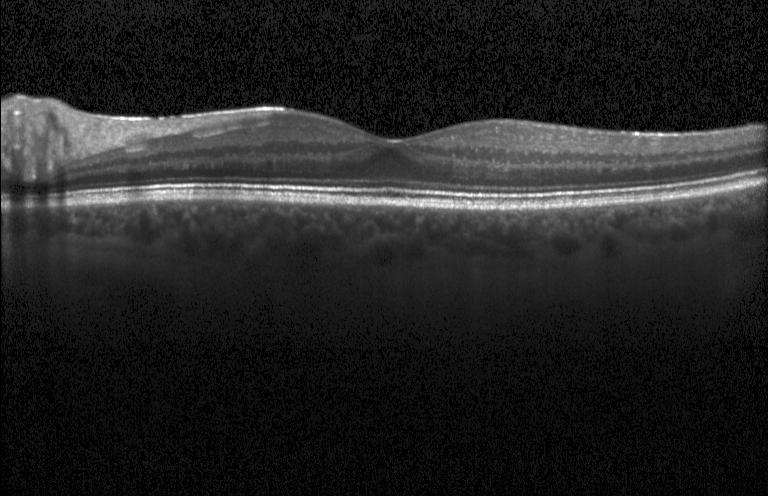

SD-OCT; horizontal scan through the fovea; optical coherence tomography B-scan; Heidelberg Spectralis OCT system. Diagnosis: neither choroidal neovascularization, diabetic macular edema, nor drusen.